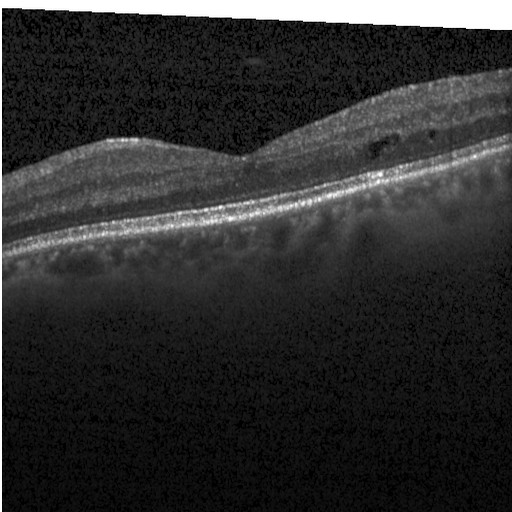 OCT finding: diabetic macular edema (DME).